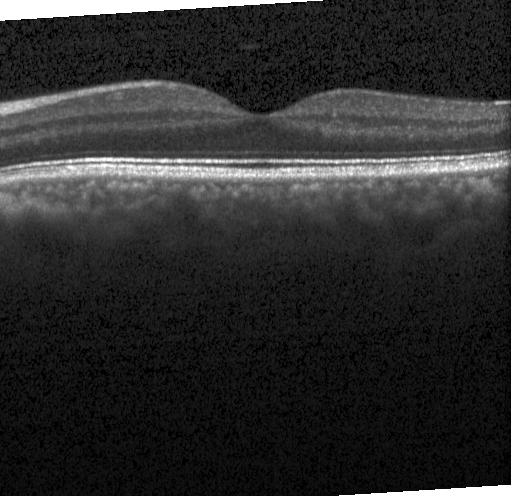

Fovea-centered, acquired on a Heidelberg Spectralis, spectral-domain OCT, OCT line scan.
Macular OCT: no evidence of CNV, DME, or drusen.